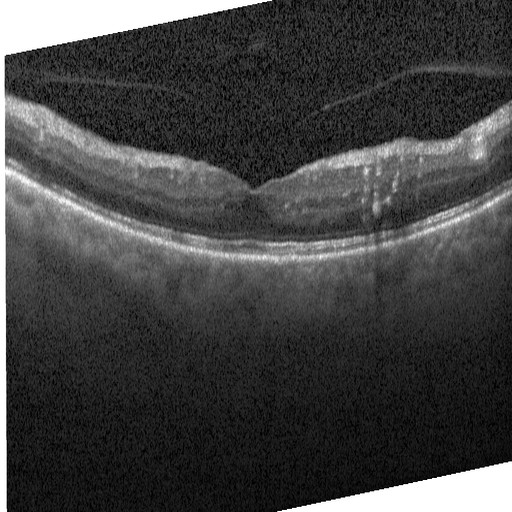
Acquired on a Heidelberg Spectralis · centered on the fovea · retinal OCT B-scan · spectral-domain optical coherence tomography
Macular OCT: diabetic macular edema.